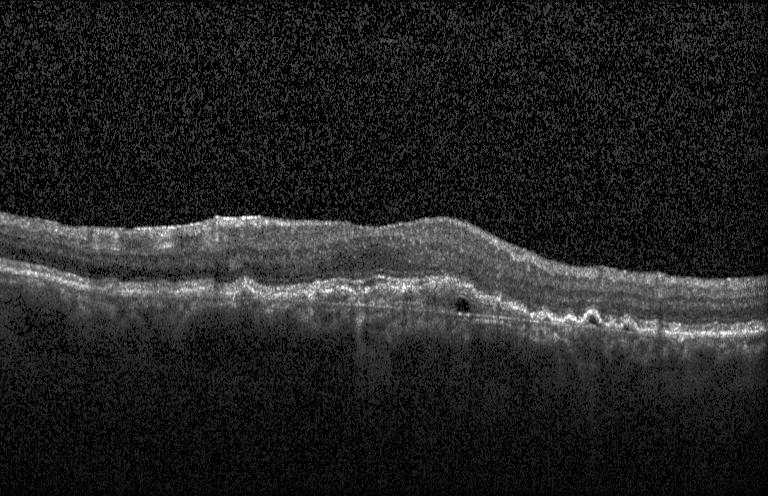 Optical coherence tomography scan · spectral-domain optical coherence tomography · instrument: Heidelberg Spectralis · centered on the fovea — OCT finding: CNV.